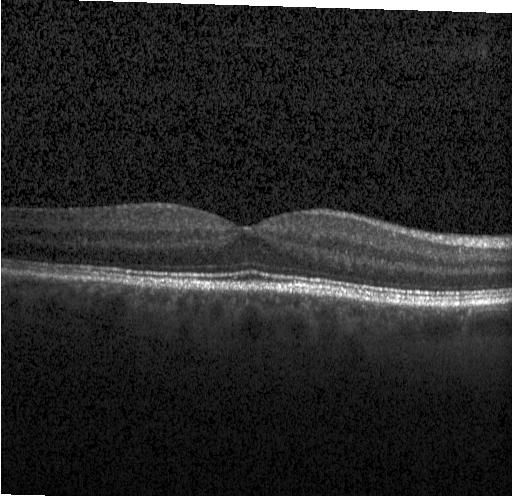 Assessment: no evidence of choroidal neovascularization, diabetic macular edema, or drusen.